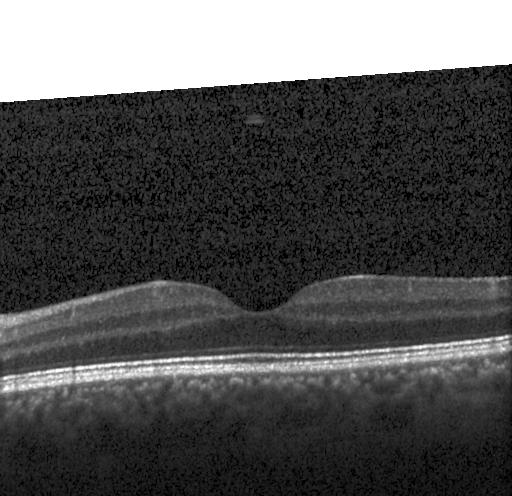 OCT B-scan
Impression: no choroidal neovascularization, diabetic macular edema, or drusen.